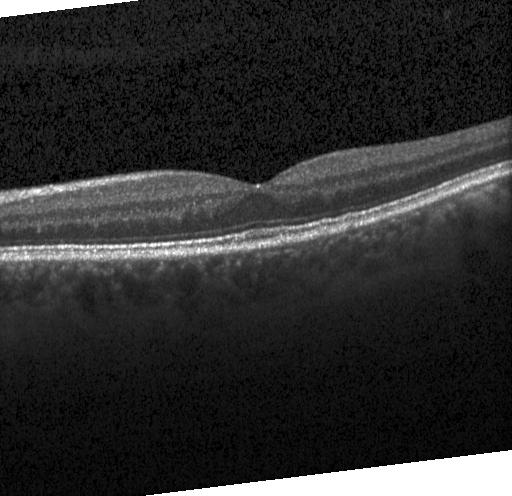

Heidelberg Spectralis. Horizontal scan through the fovea. Optical coherence tomography scan — Diagnosis: no evidence of choroidal neovascularization, diabetic macular edema, or drusen.